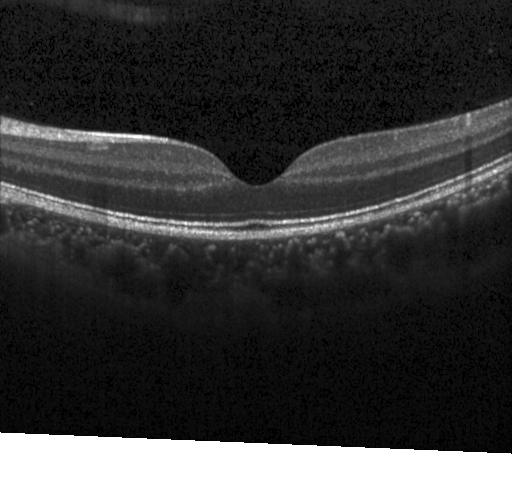
Diagnosis: no CNV, DME, or drusen.